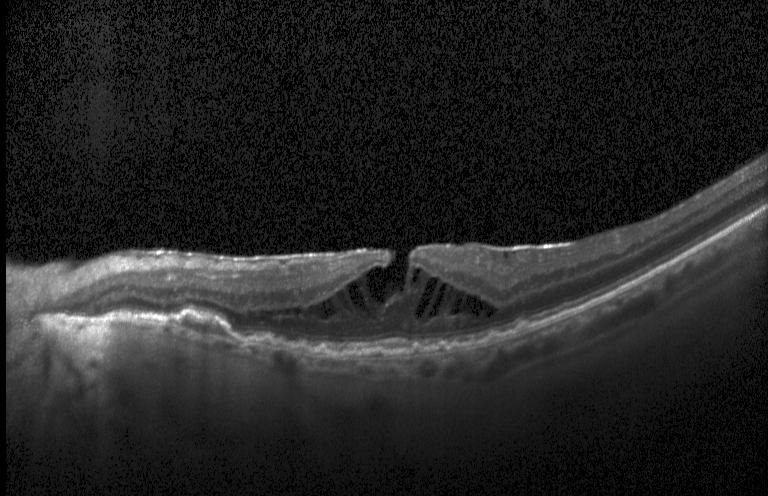

Heidelberg Spectralis; spectral-domain OCT; fovea-centered; OCT B-scan — Finding: diabetic macular edema.